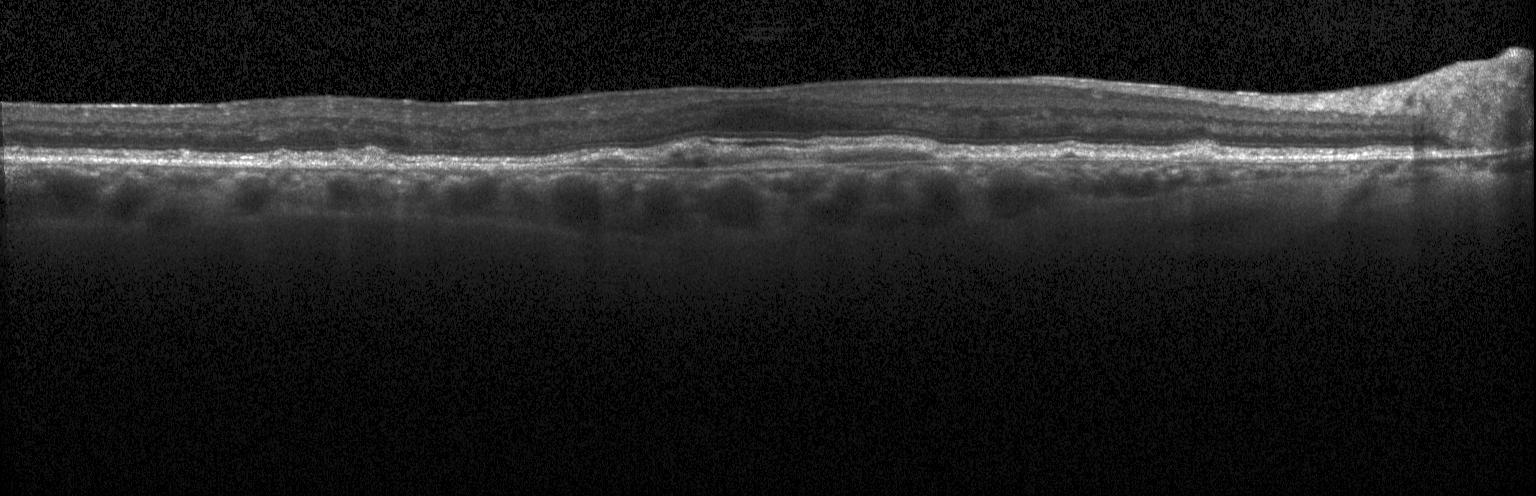

Heidelberg Spectralis, retinal OCT B-scan, spectral-domain optical coherence tomography. Impression: CNV.